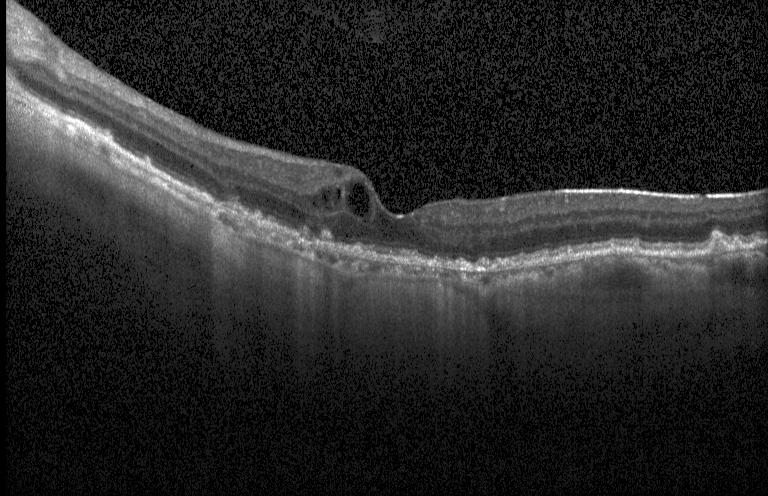

Retinal OCT cross-section.
The scan shows a choroidal neovascular membrane.